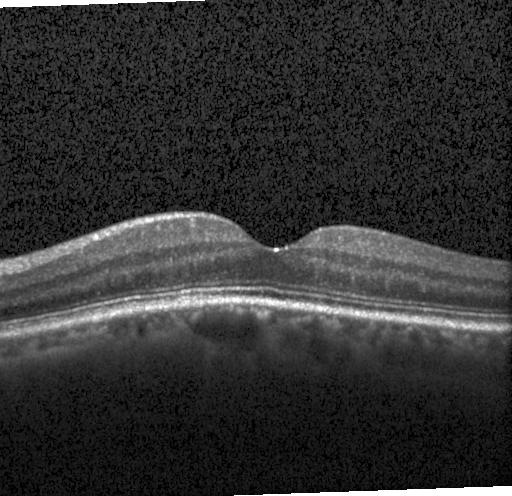 OCT line scan · centered on the fovea · spectral-domain optical coherence tomography · Heidelberg Spectralis.
This B-scan demonstrates no evidence of choroidal neovascularization, diabetic macular edema, or drusen.